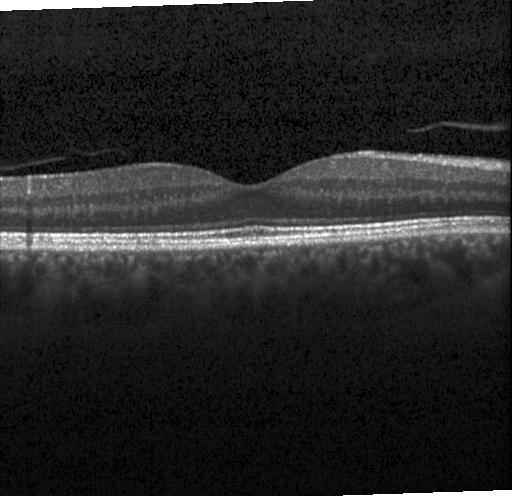 Macular OCT: no evidence of CNV, DME, or drusen.